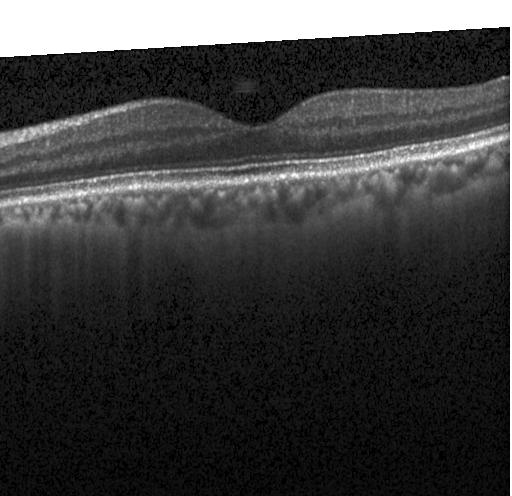
Centered on the fovea · retinal OCT cross-section · spectral-domain OCT · instrument: Heidelberg Spectralis. This B-scan demonstrates neither CNV, DME, nor drusen.